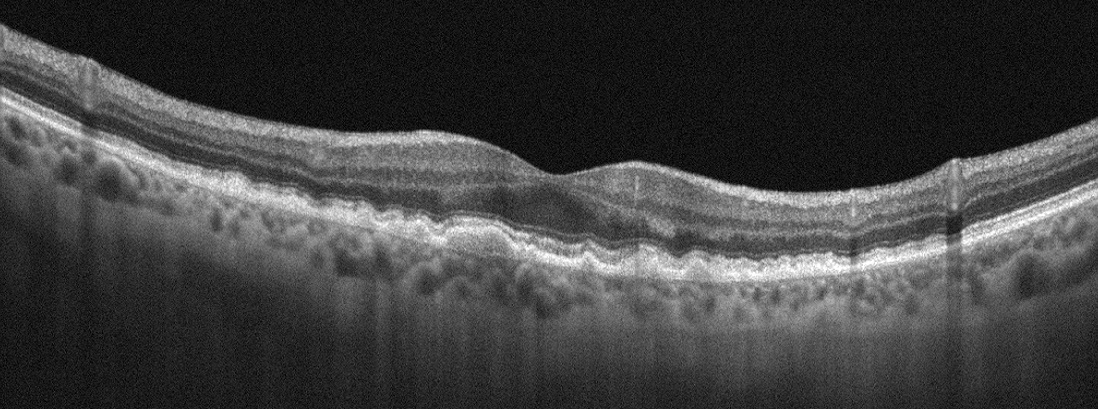

Through the macula; retinal OCT B-scan — Finding: age-related macular degeneration.